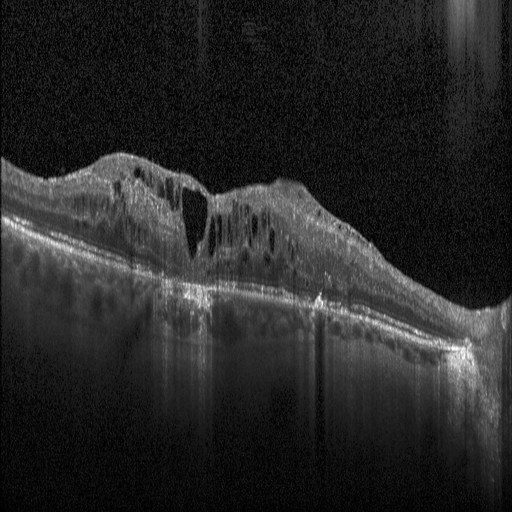

Optical coherence tomography B-scan; fovea-centered; instrument: Heidelberg Spectralis; spectral-domain OCT. Finding: diabetic macular edema (DME).